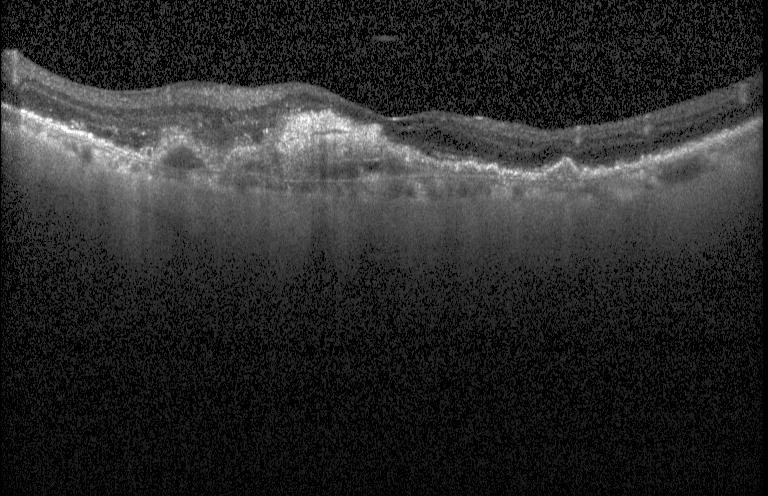

OCT scan showing a choroidal neovascular membrane.